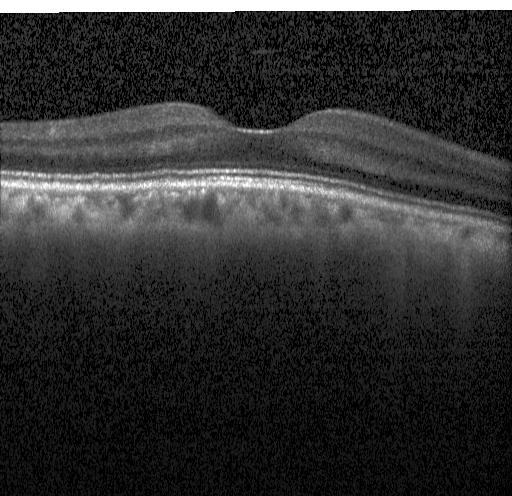 Retinal OCT B-scan — Impression: no evidence of choroidal neovascularization, diabetic macular edema, or drusen.